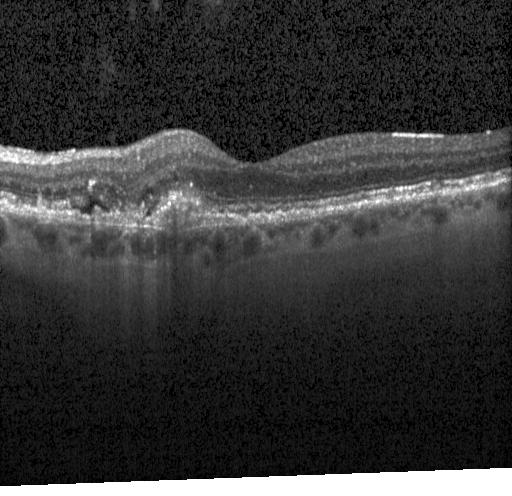 Heidelberg Spectralis OCT system, SD-OCT, retinal OCT cross-section
Finding: choroidal neovascularization.